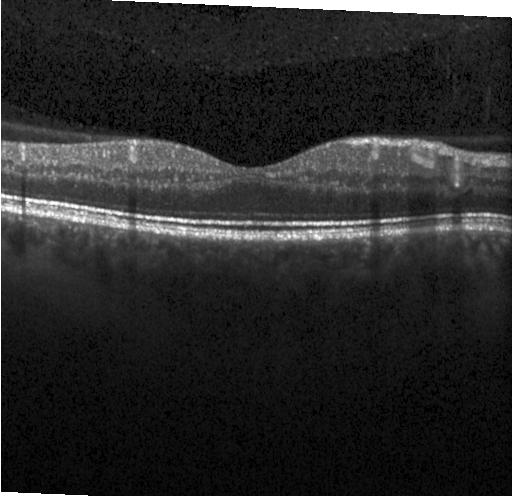

This B-scan demonstrates no choroidal neovascularization, no diabetic macular edema, and no drusen.